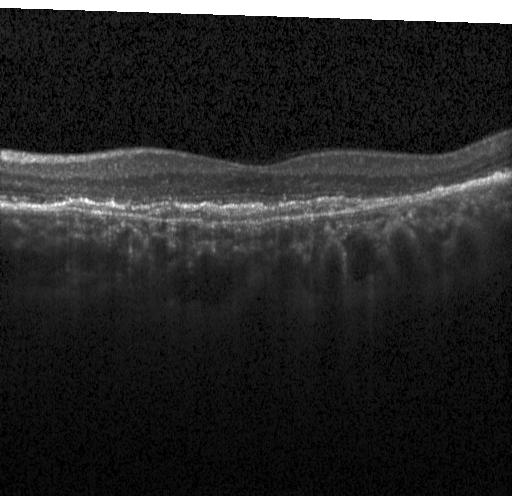
Impression: CNV.